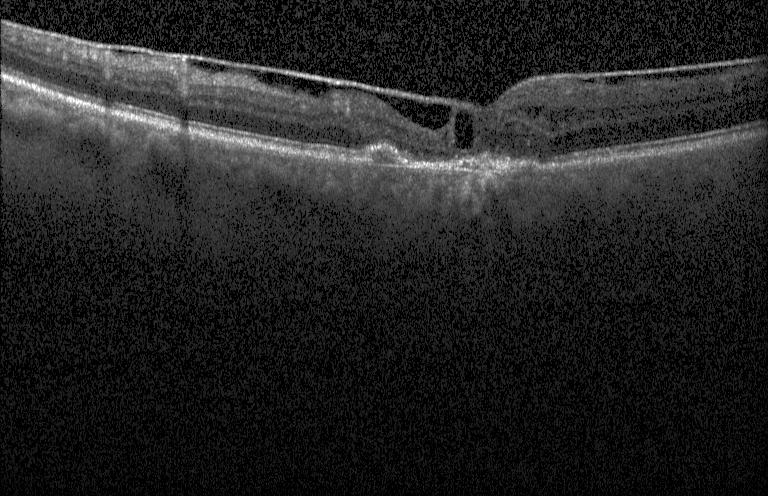 Horizontal scan through the fovea, OCT B-scan. The scan shows choroidal neovascularization (CNV).